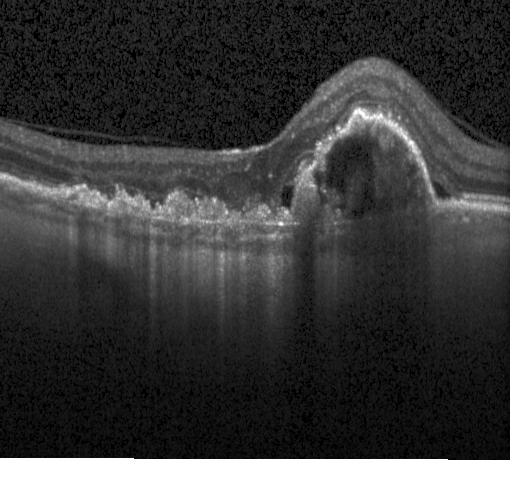 OCT B-scan
Impression: a choroidal neovascular membrane.